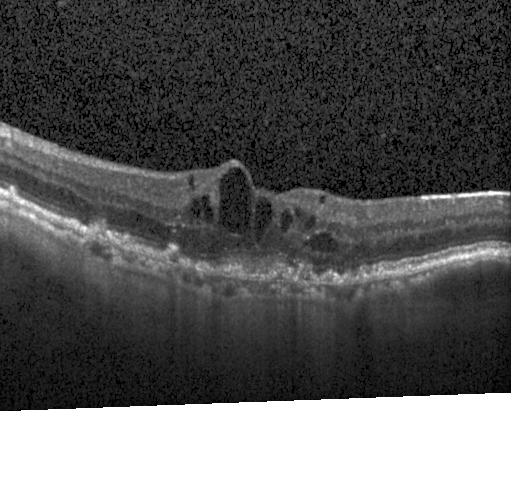

Diagnosis: choroidal neovascularization (CNV).